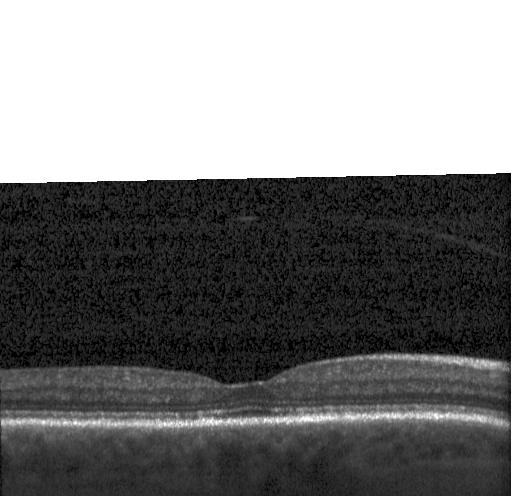

Retinal OCT B-scan
Impression: no choroidal neovascularization, diabetic macular edema, or drusen.